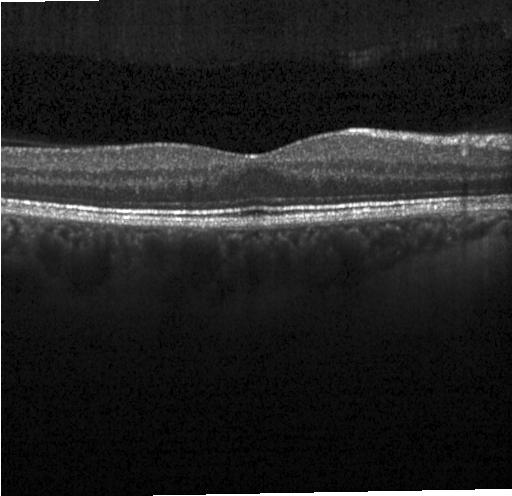 Heidelberg Spectralis. Retinal OCT B-scan. Spectral-domain OCT. Horizontal scan through the fovea — Finding: neither choroidal neovascularization, diabetic macular edema, nor drusen.